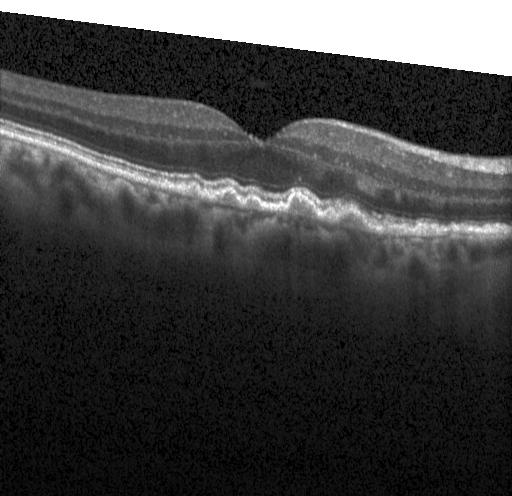
Optical coherence tomography B-scan. Heidelberg Spectralis. Spectral-domain optical coherence tomography. Fovea-centered
This B-scan demonstrates sub-RPE drusenoid deposits.